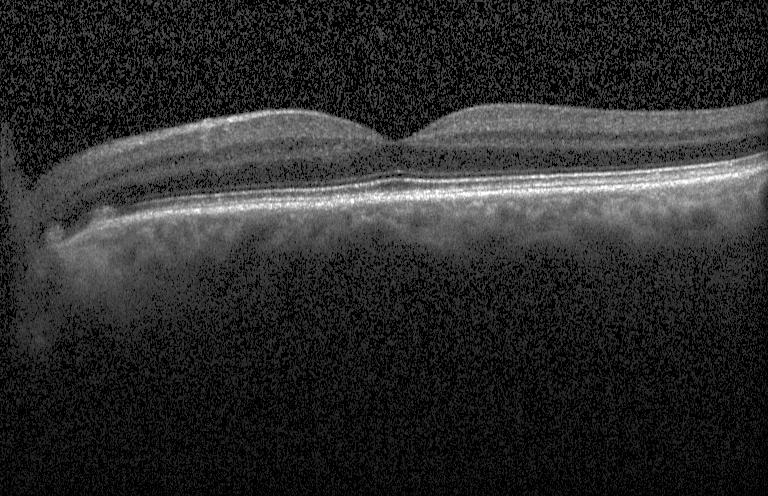
Dx: no evidence of CNV, DME, or drusen.